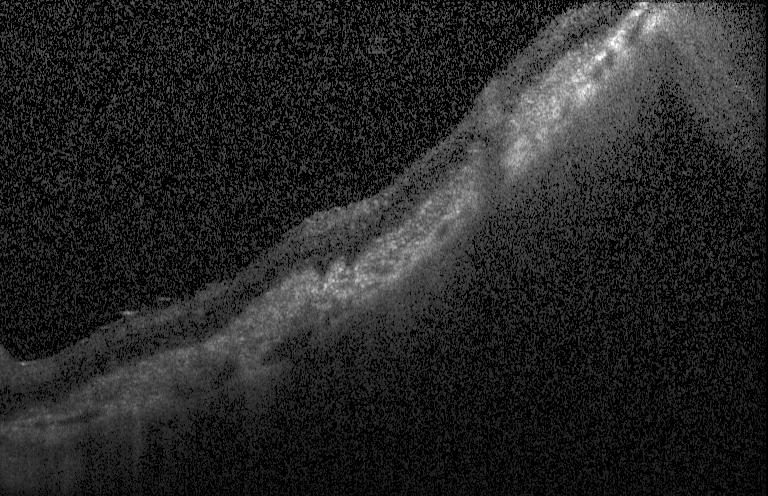
Assessment: a choroidal neovascular membrane.